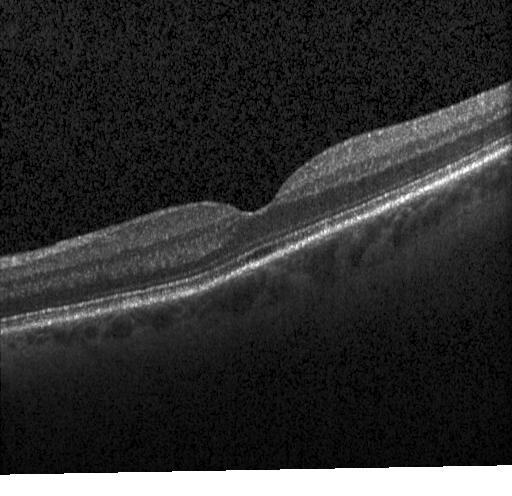
Optical coherence tomography B-scan, horizontal scan through the fovea — The scan shows no evidence of CNV, DME, or drusen.